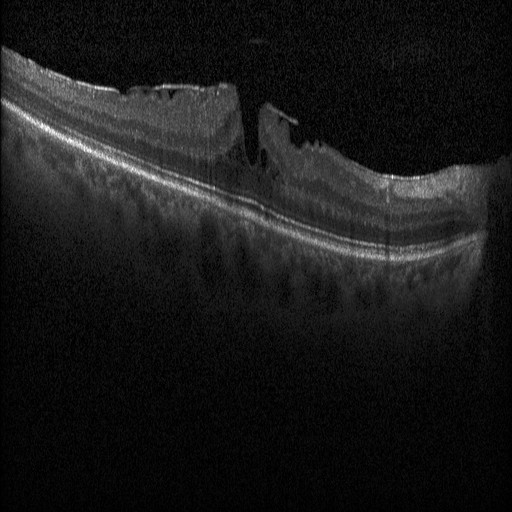

OCT B-scan, SD-OCT
Finding: DME.